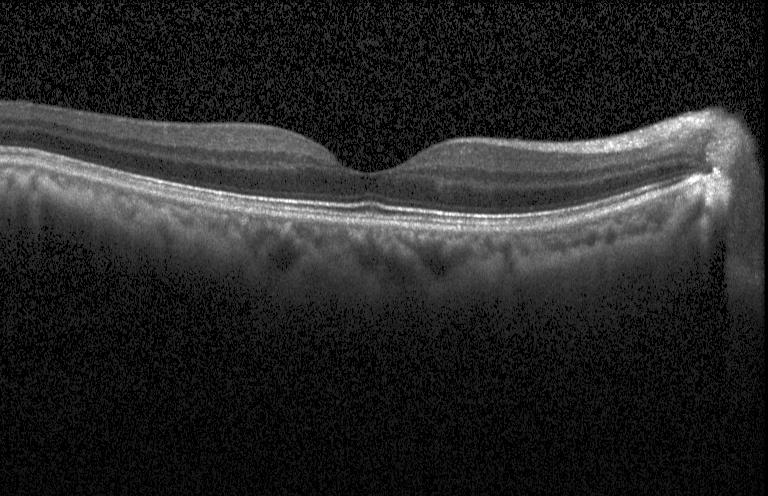 Macular OCT: no evidence of CNV, DME, or drusen.